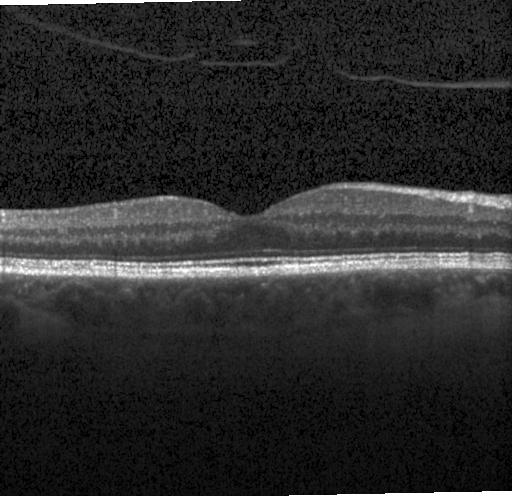 Heidelberg Spectralis, fovea-centered, optical coherence tomography scan. This B-scan demonstrates neither CNV, DME, nor drusen.